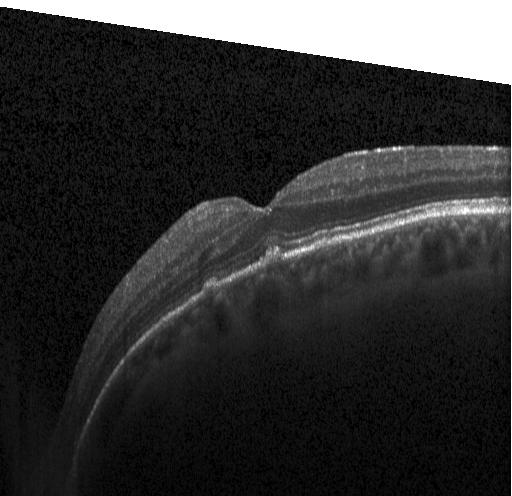
Spectral-domain OCT B-scan: drusen.